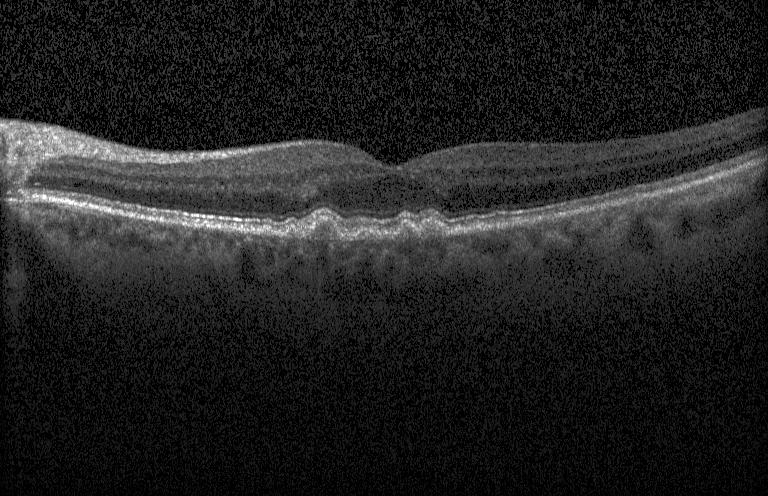

This B-scan demonstrates multiple drusen.